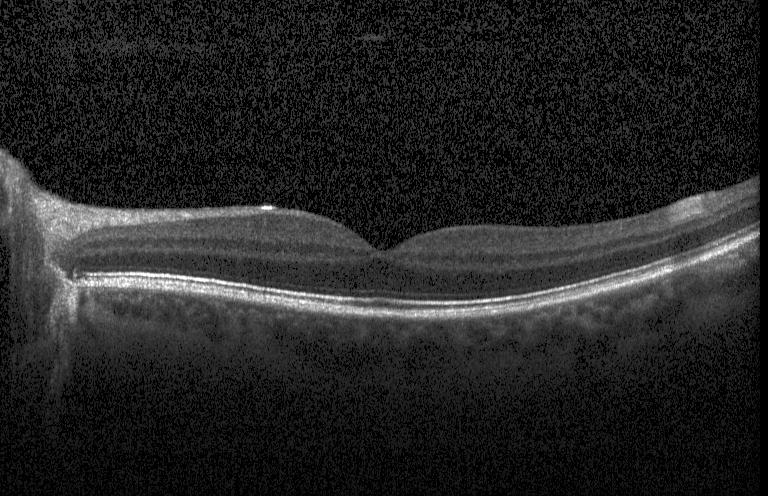 OCT line scan; SD-OCT; instrument: Heidelberg Spectralis; macular scan. The scan shows neither choroidal neovascularization, diabetic macular edema, nor drusen.